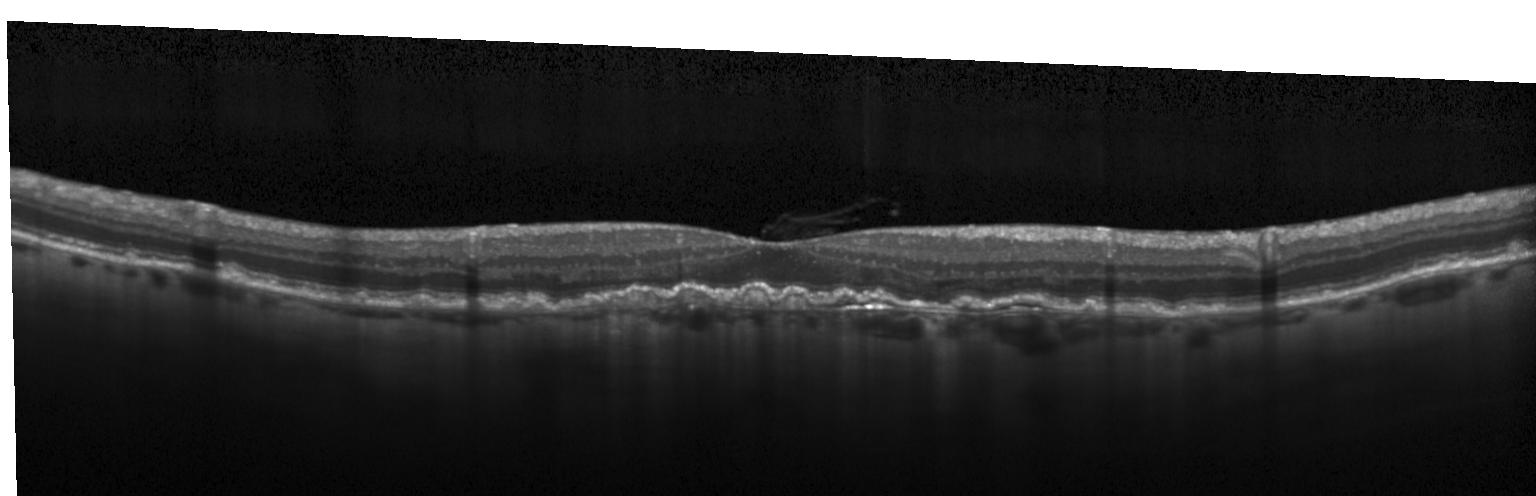

Impression: choroidal neovascularization.